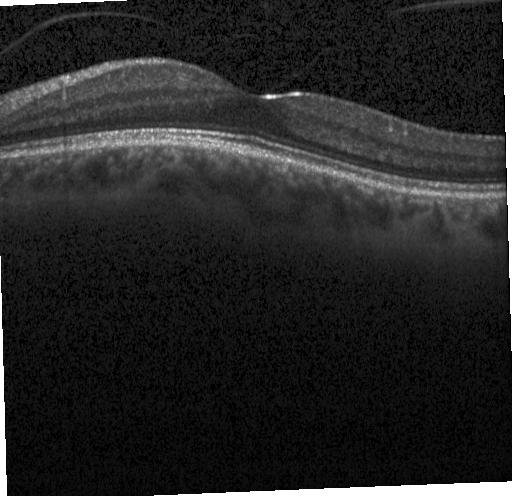 No evidence of choroidal neovascularization, diabetic macular edema, or drusen.